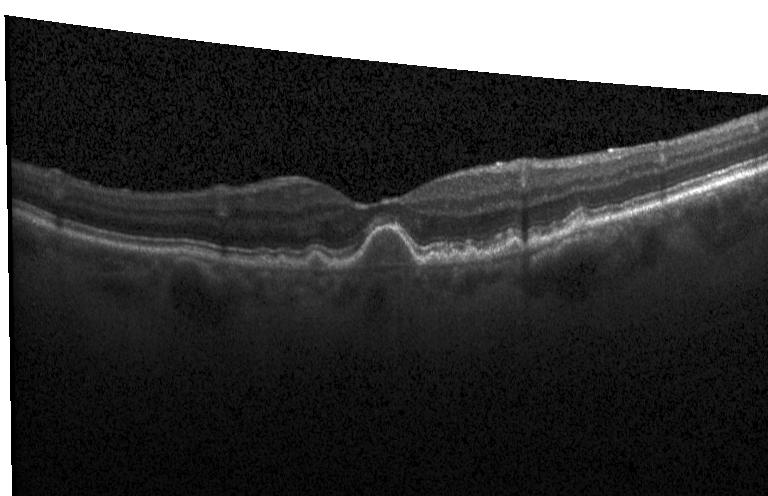
Sub-RPE drusenoid deposits.